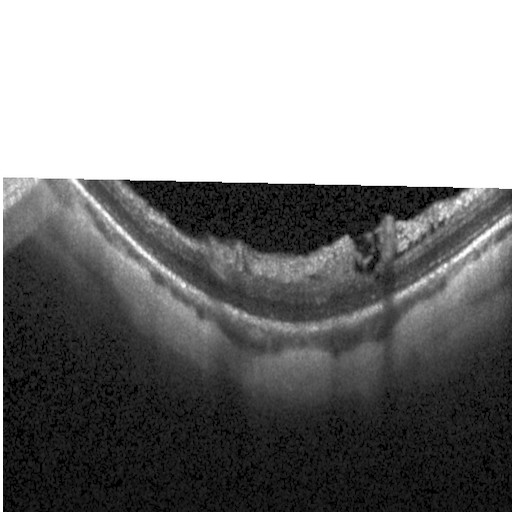 Centered on the fovea · Heidelberg Spectralis OCT system · retinal OCT cross-section · SD-OCT
OCT finding: DME.